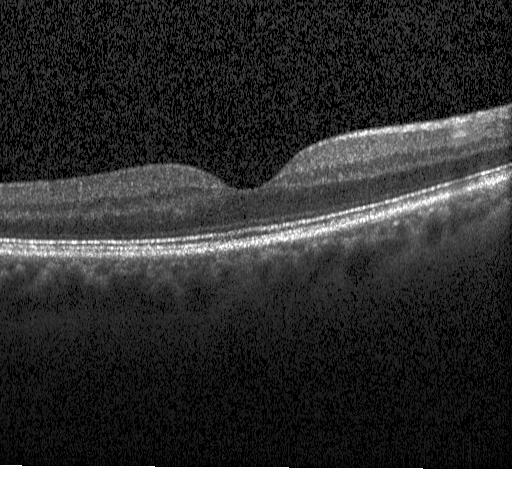

Retinal OCT cross-section showing neither choroidal neovascularization, diabetic macular edema, nor drusen.